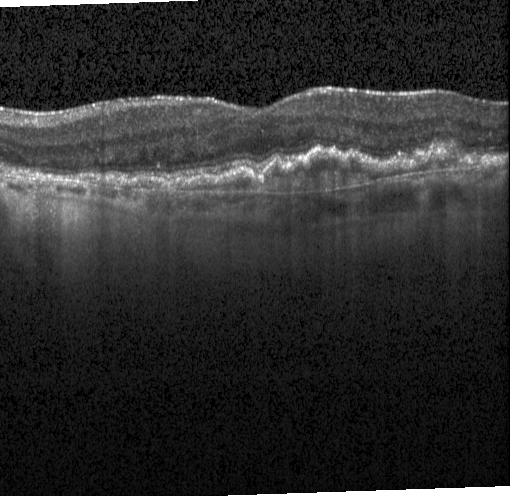

Finding: a choroidal neovascular membrane.